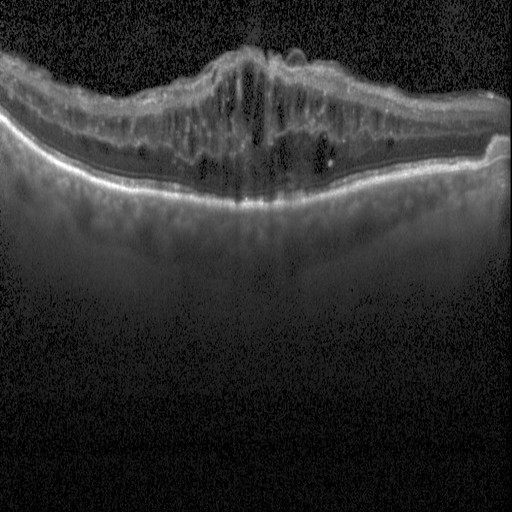 Spectral-domain OCT B-scan: diabetic macular edema.